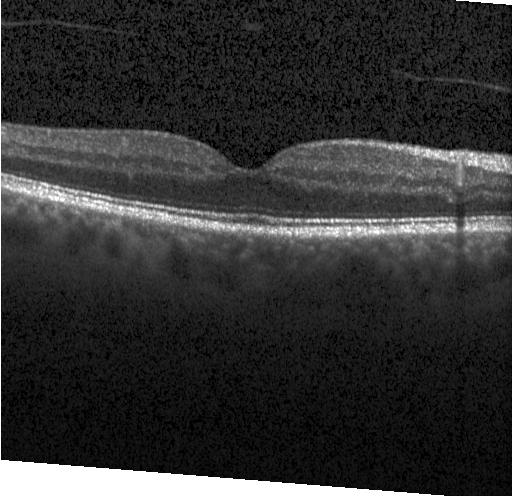

Finding: no choroidal neovascularization, no diabetic macular edema, and no drusen.